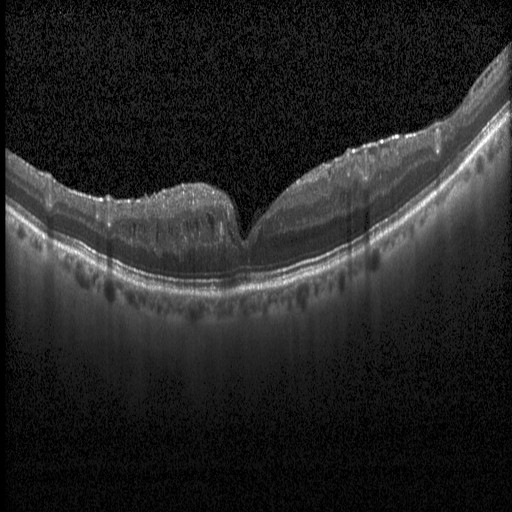 Impression: diabetic macular edema.